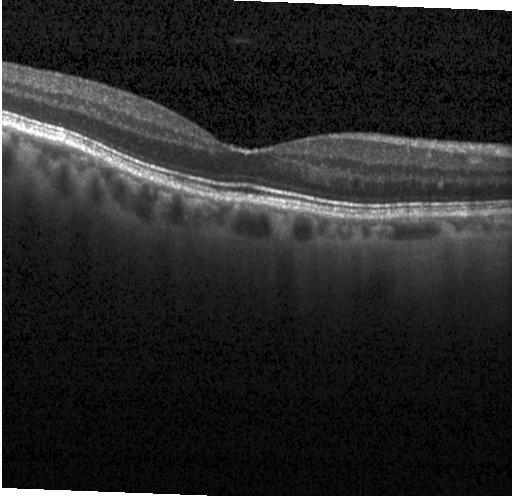
Instrument: Heidelberg Spectralis; spectral-domain optical coherence tomography; OCT line scan; through the macula. No choroidal neovascularization, diabetic macular edema, or drusen.